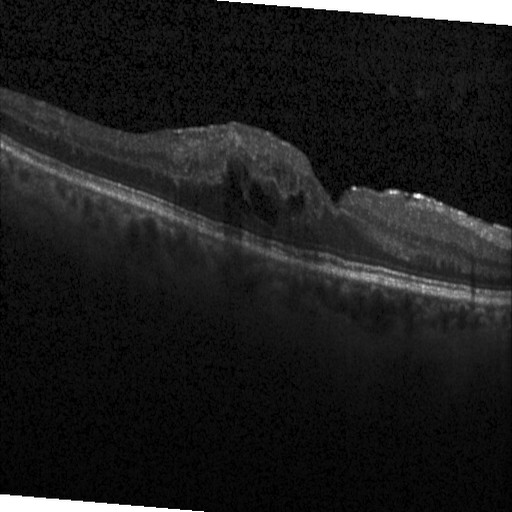
Assessment: diabetic macular edema.